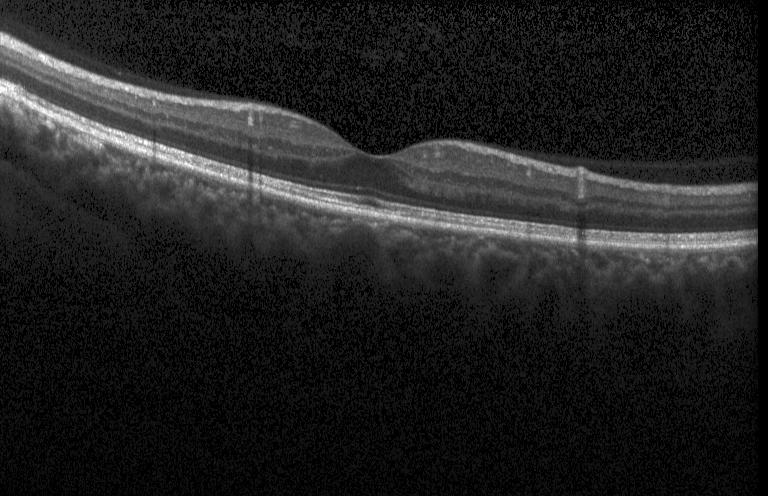 OCT finding: no evidence of CNV, DME, or drusen.